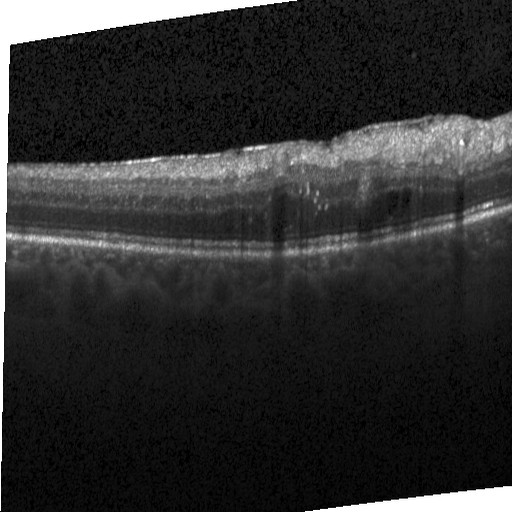 Instrument: Heidelberg Spectralis, SD-OCT, retinal OCT cross-section. The scan shows diabetic macular edema.